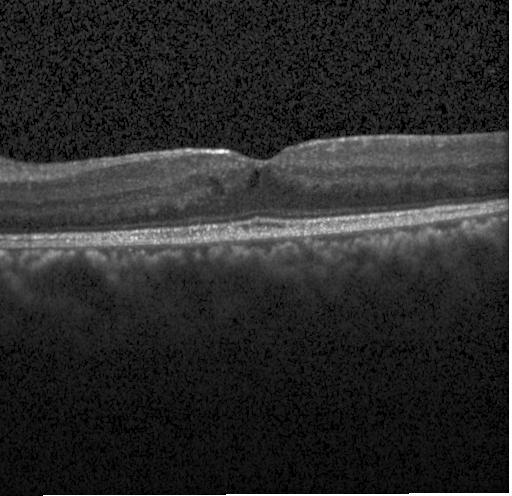

Horizontal scan through the fovea; SD-OCT; retinal OCT B-scan — Diagnosis: DME.